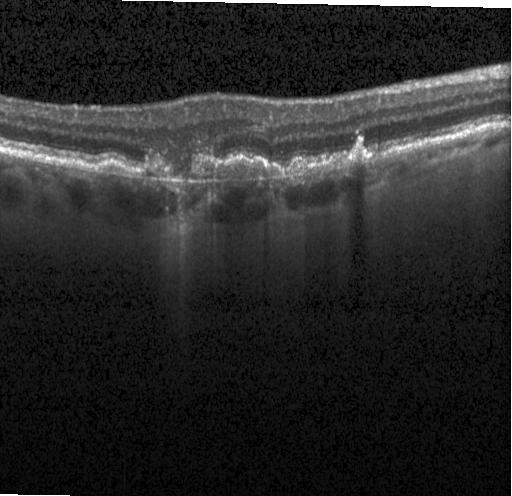 OCT line scan, fovea-centered. The scan shows choroidal neovascularization (CNV).